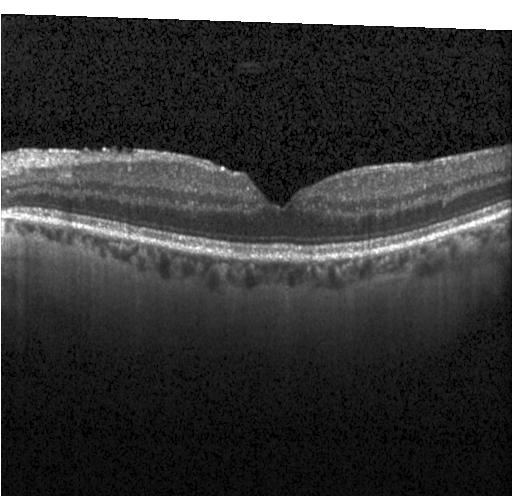

Impression: no choroidal neovascularization, diabetic macular edema, or drusen.